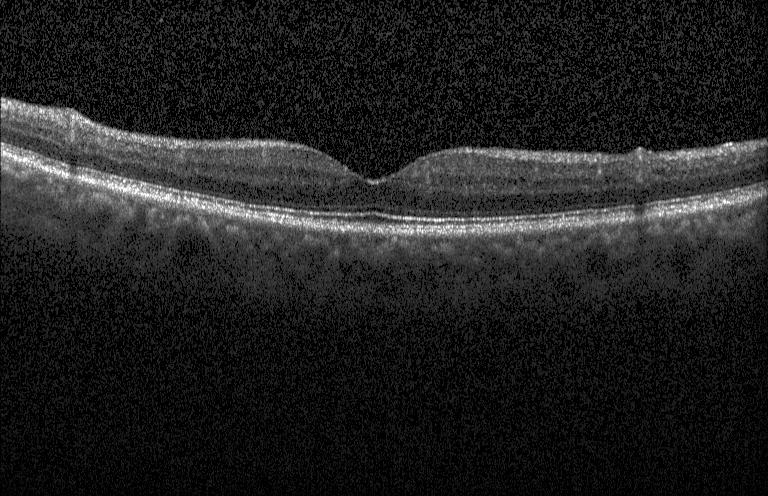 Spectral-domain OCT B-scan: no CNV, DME, or drusen.